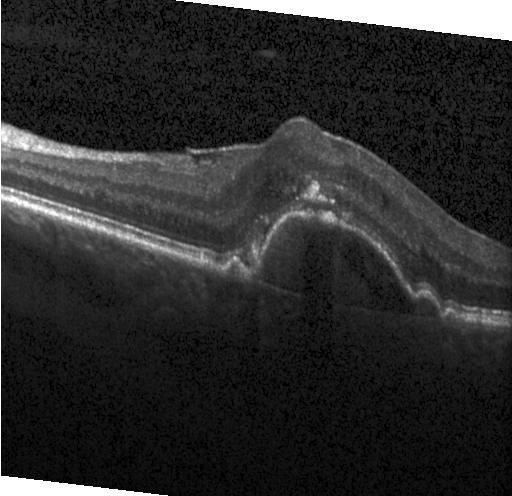 Retinal OCT cross-section showing choroidal neovascularization.